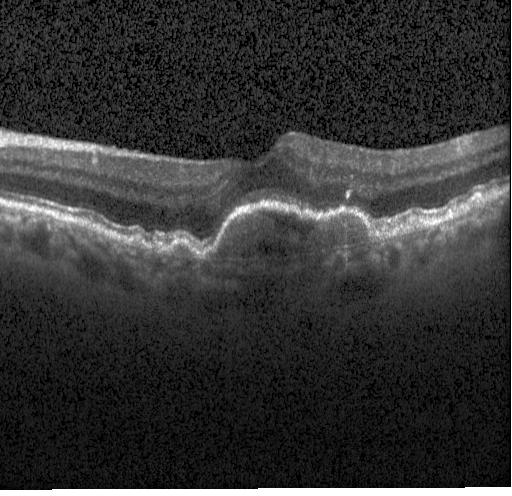

Retinal OCT cross-section.
This B-scan demonstrates drusen.